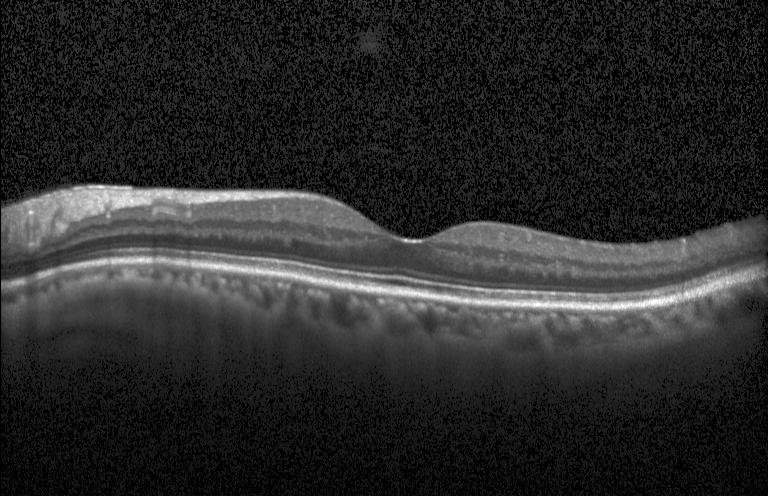 Diagnosis: neither choroidal neovascularization, diabetic macular edema, nor drusen.